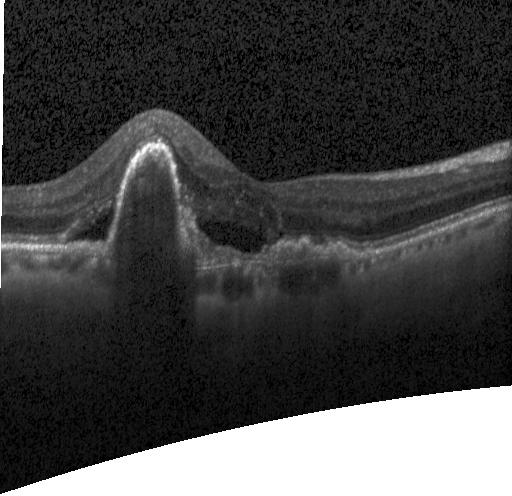

Spectral-domain OCT B-scan: CNV.